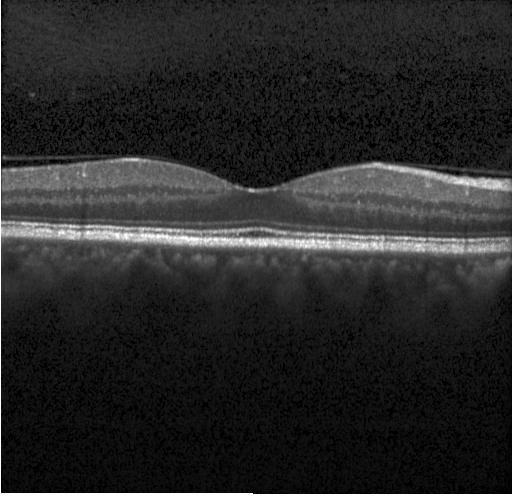 Impression: neither choroidal neovascularization, diabetic macular edema, nor drusen.